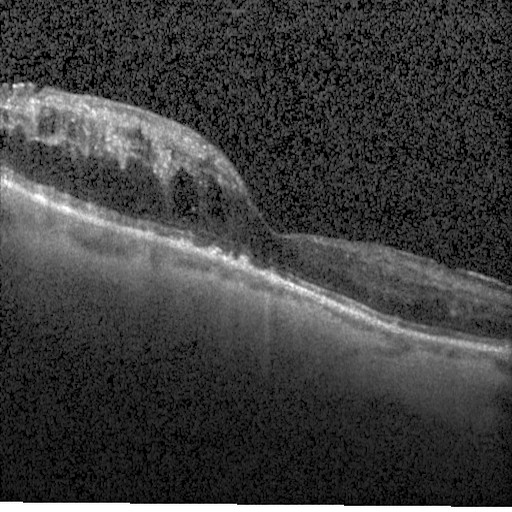
Finding: DME.